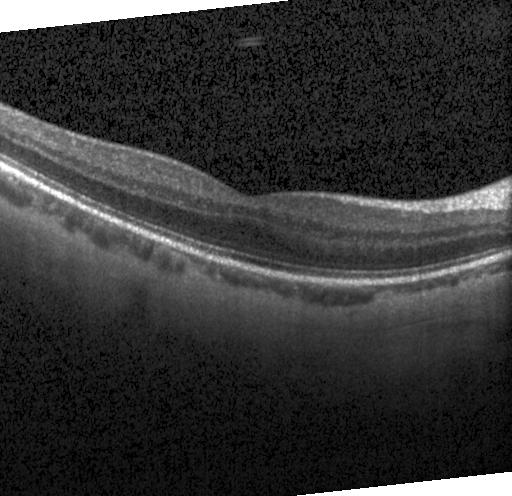 Optical coherence tomography B-scan. Impression: no CNV, no DME, and no drusen.